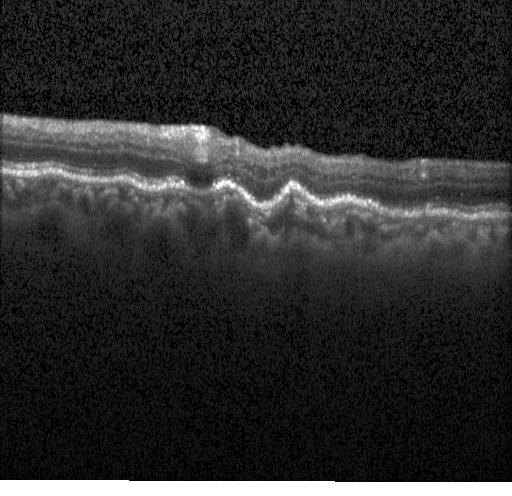

Dx: a choroidal neovascular membrane.